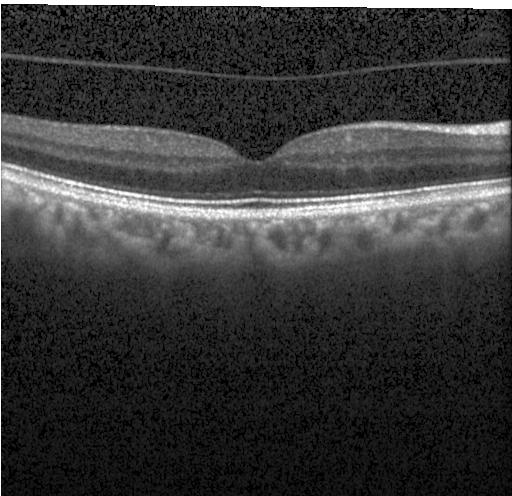
Diagnosis: no CNV, DME, or drusen.